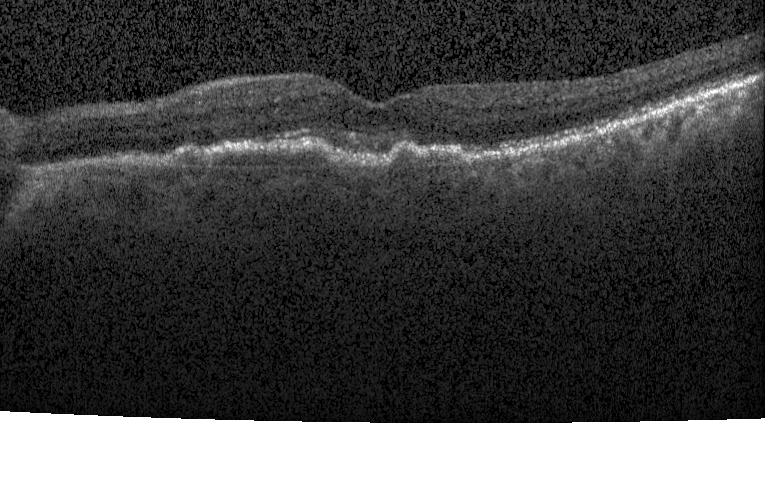
Diagnosis: a choroidal neovascular membrane.